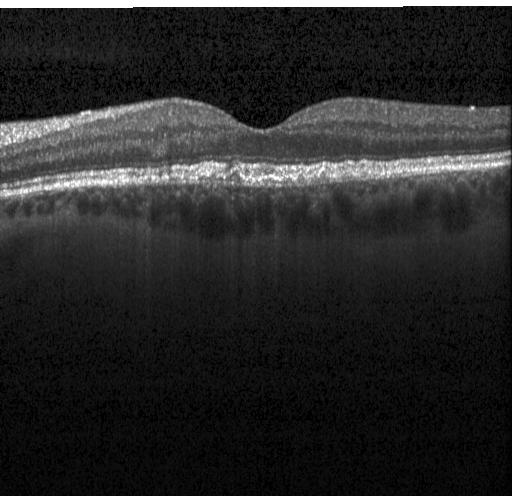 Retinal OCT cross-section — Dx: drusen.